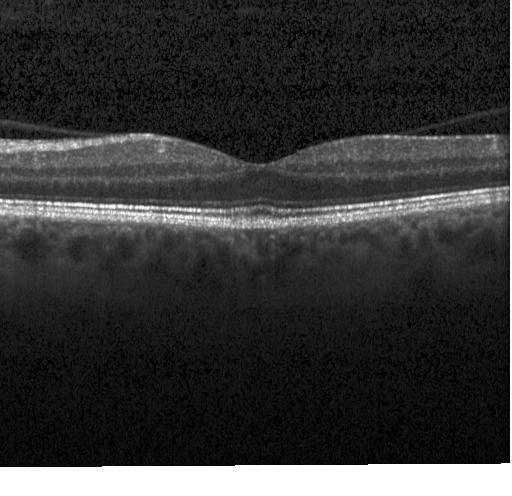 Centered on the fovea · spectral-domain OCT · retinal OCT cross-section · instrument: Heidelberg Spectralis
No evidence of CNV, DME, or drusen.